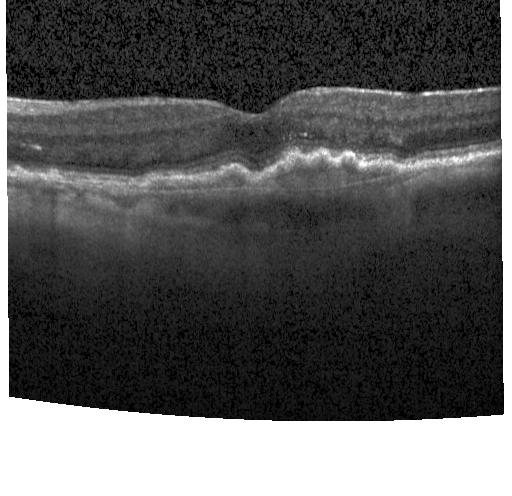
Spectral-domain OCT. Retinal OCT B-scan. Fovea-centered. Instrument: Heidelberg Spectralis. Finding: a choroidal neovascular membrane.